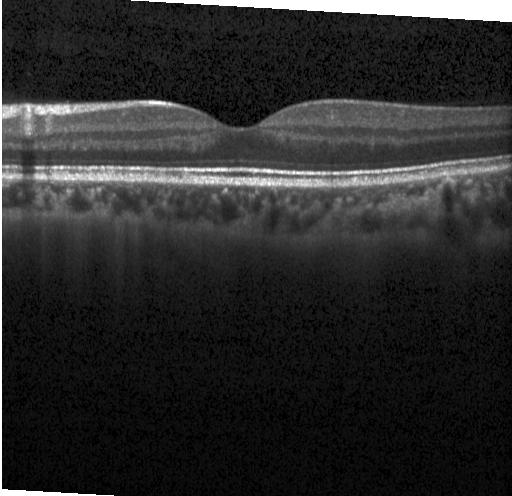
Dx: no evidence of choroidal neovascularization, diabetic macular edema, or drusen.